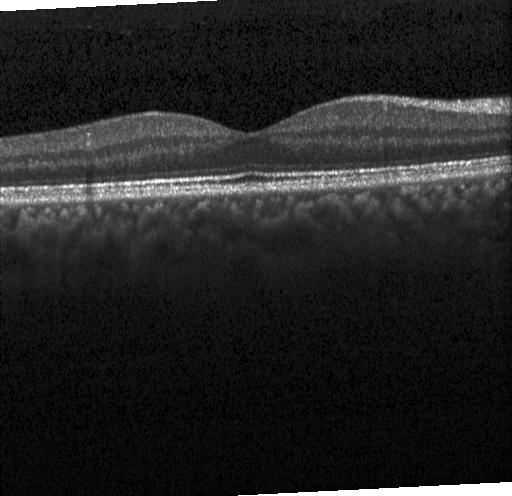
SD-OCT, instrument: Heidelberg Spectralis, horizontal scan through the fovea, optical coherence tomography B-scan — The scan shows neither choroidal neovascularization, diabetic macular edema, nor drusen.